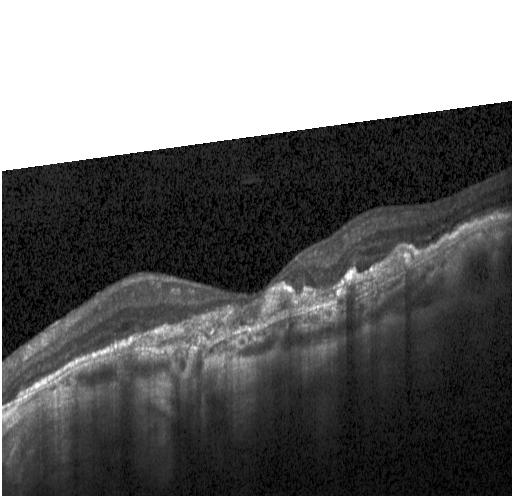 OCT line scan, macular scan
Diagnosis: a choroidal neovascular membrane.